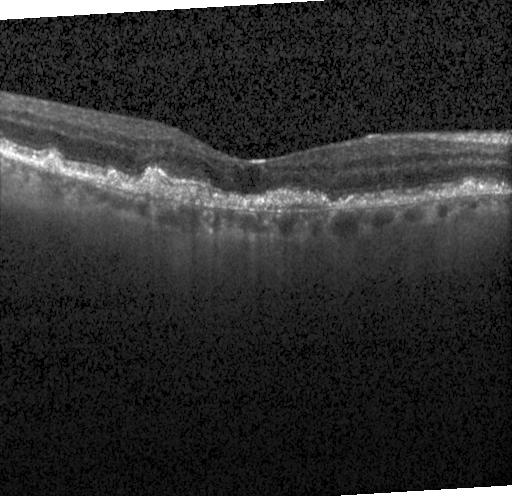 Diagnosis: a choroidal neovascular membrane.